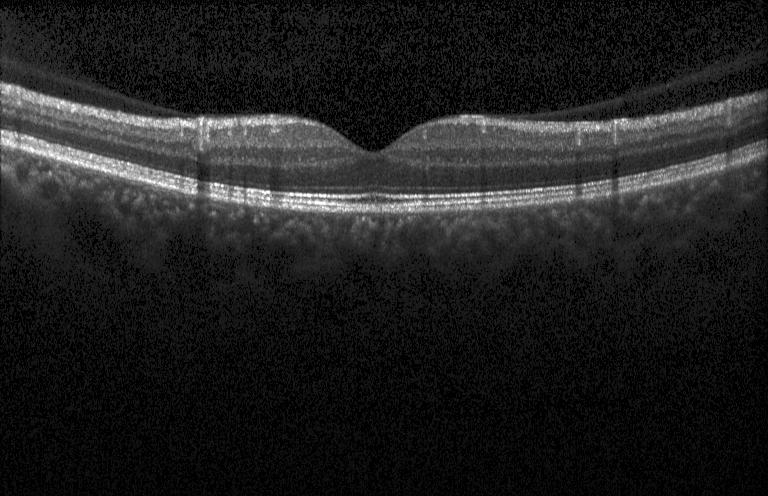
OCT B-scan showing no evidence of choroidal neovascularization, diabetic macular edema, or drusen.